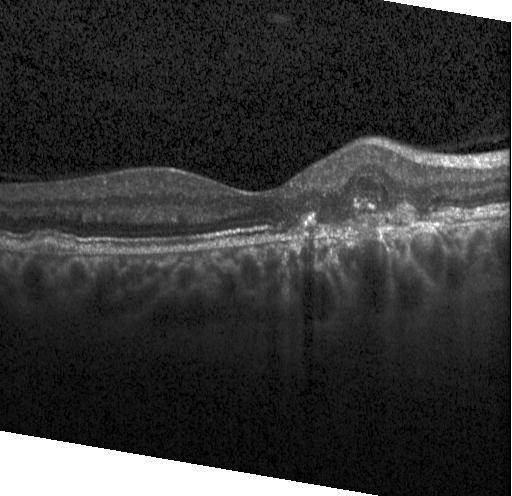
Heidelberg Spectralis · retinal OCT cross-section · spectral-domain OCT
OCT finding: choroidal neovascularization.